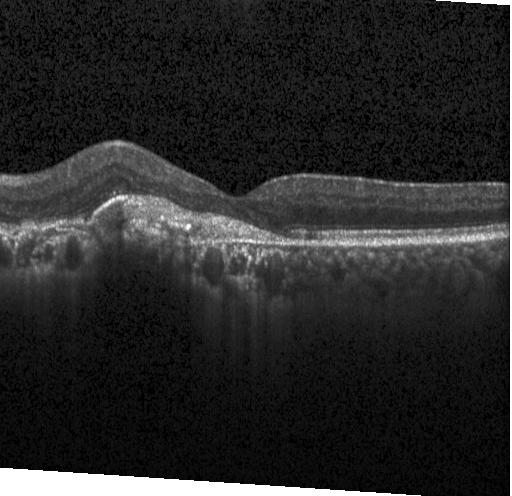

Finding: choroidal neovascularization.